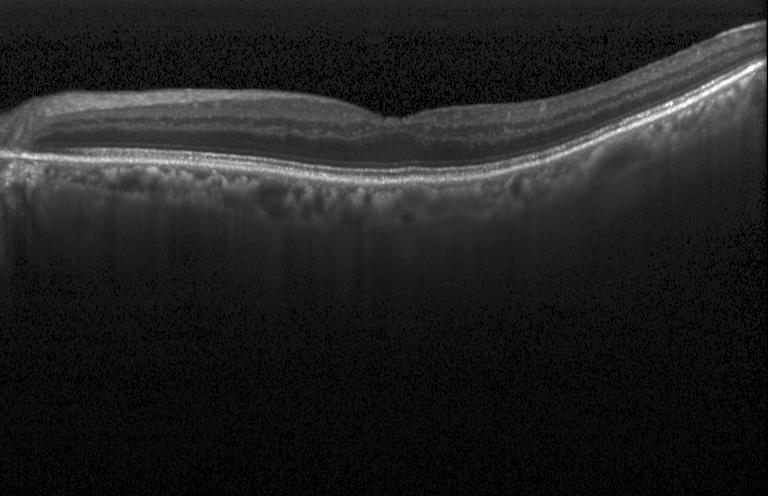

Finding: no CNV, DME, or drusen.